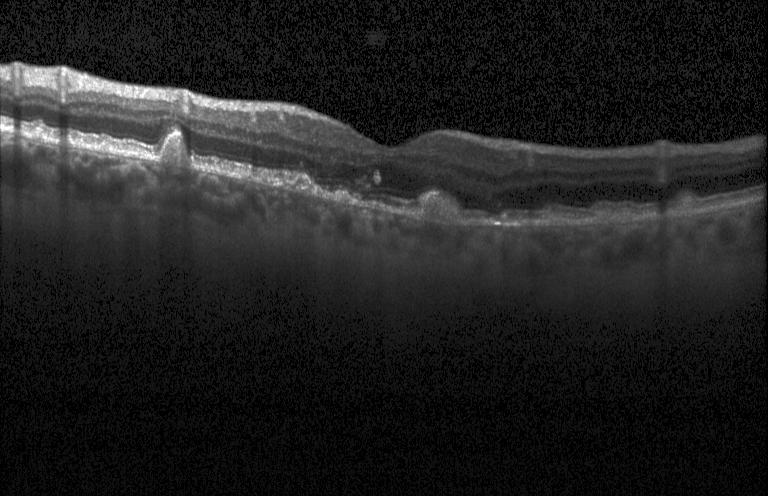
Instrument: Heidelberg Spectralis; OCT line scan; SD-OCT. Drusen.